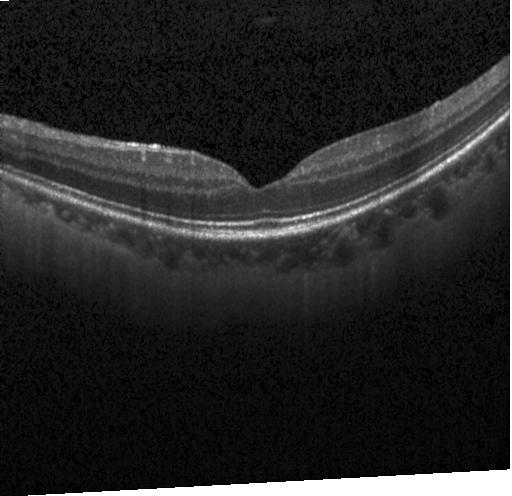
Diagnosis: no evidence of choroidal neovascularization, diabetic macular edema, or drusen.